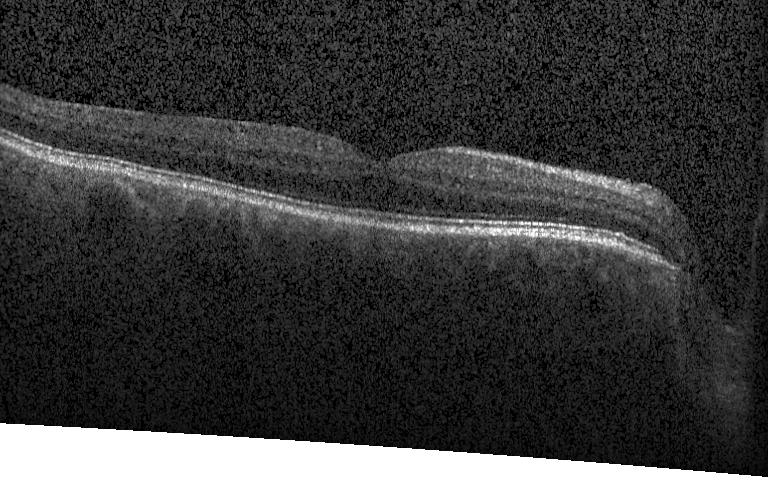 Spectral-domain optical coherence tomography; retinal OCT B-scan; horizontal scan through the fovea; Heidelberg Spectralis OCT system — This B-scan demonstrates no evidence of choroidal neovascularization, diabetic macular edema, or drusen.